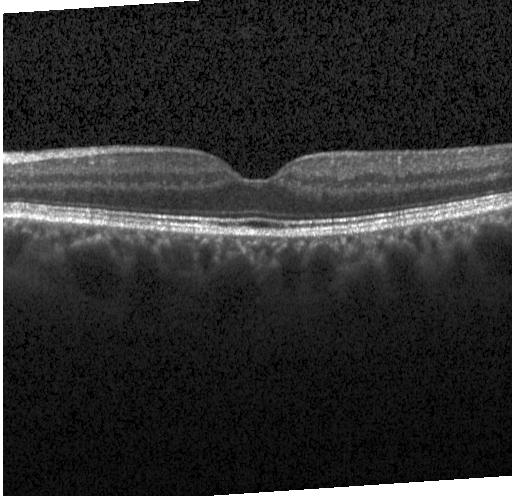

Retinal OCT B-scan; centered on the fovea. Assessment: no choroidal neovascularization, diabetic macular edema, or drusen.